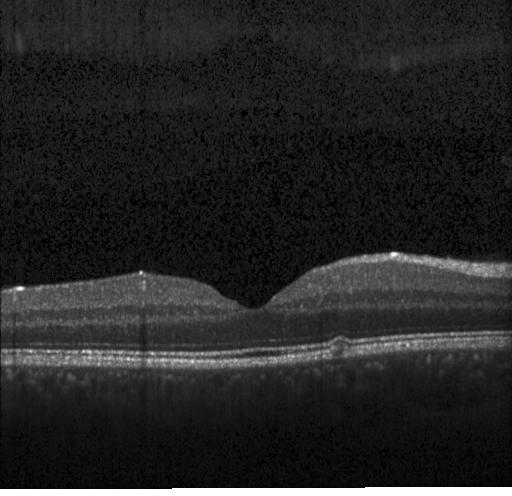

Retinal OCT B-scan
The scan shows neither choroidal neovascularization, diabetic macular edema, nor drusen.